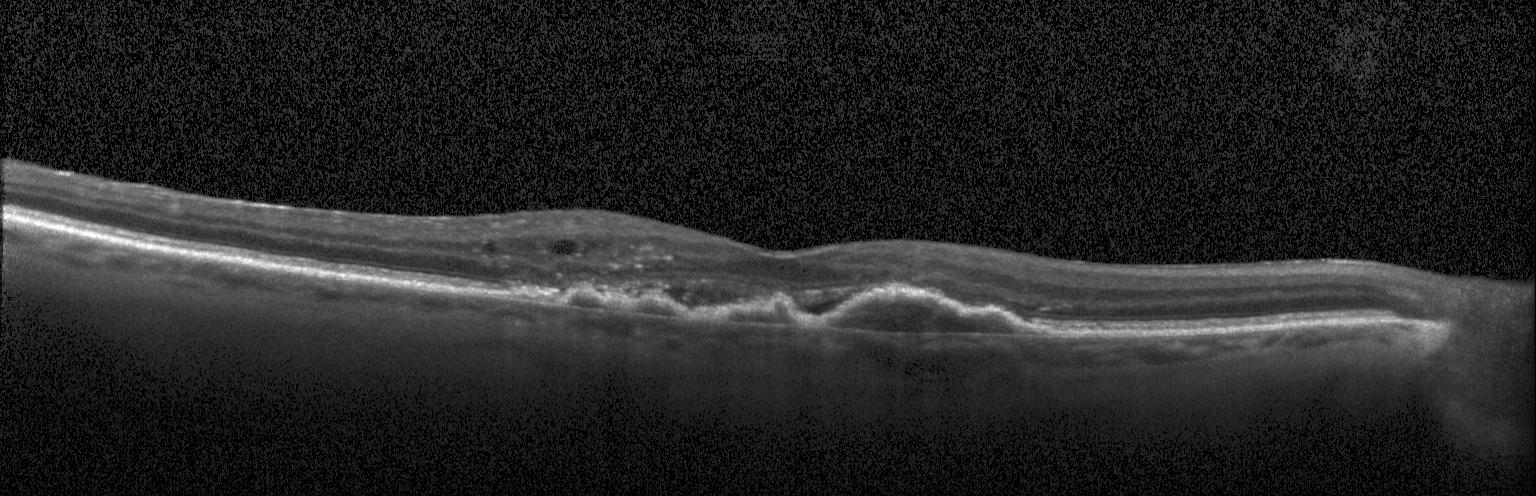 OCT B-scan showing CNV.